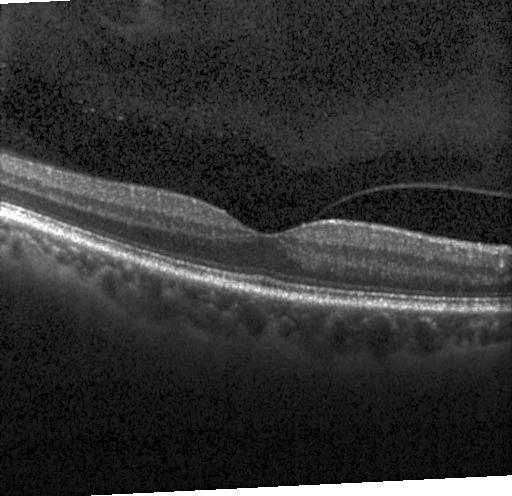
Retinal OCT cross-section.
No choroidal neovascularization, no diabetic macular edema, and no drusen.